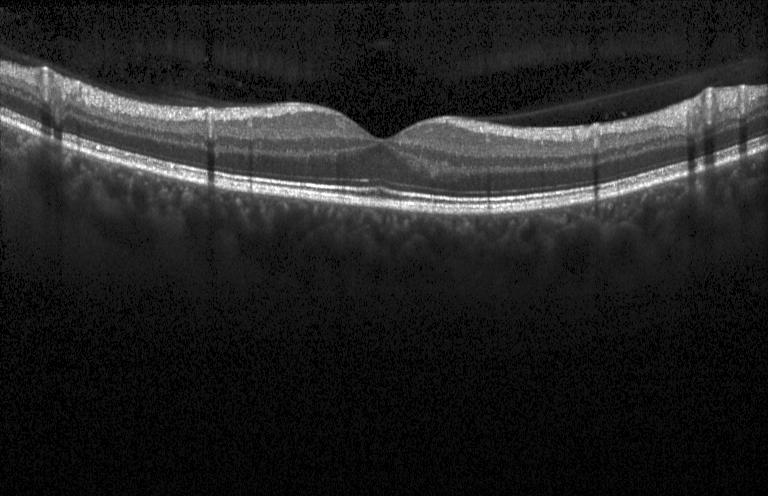
Optical coherence tomography B-scan · spectral-domain OCT · horizontal scan through the fovea · Heidelberg Spectralis OCT system.
Finding: no choroidal neovascularization, no diabetic macular edema, and no drusen.